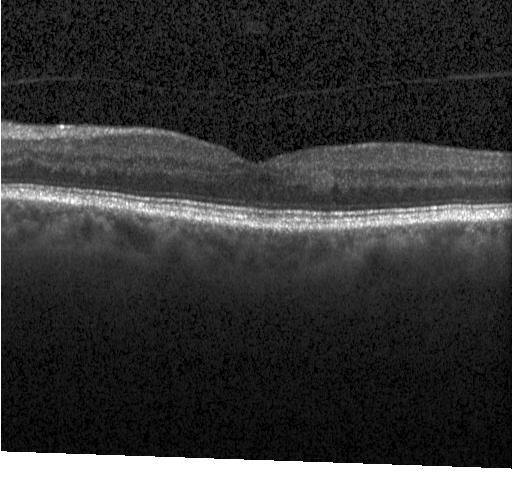 Assessment: no CNV, no DME, and no drusen.